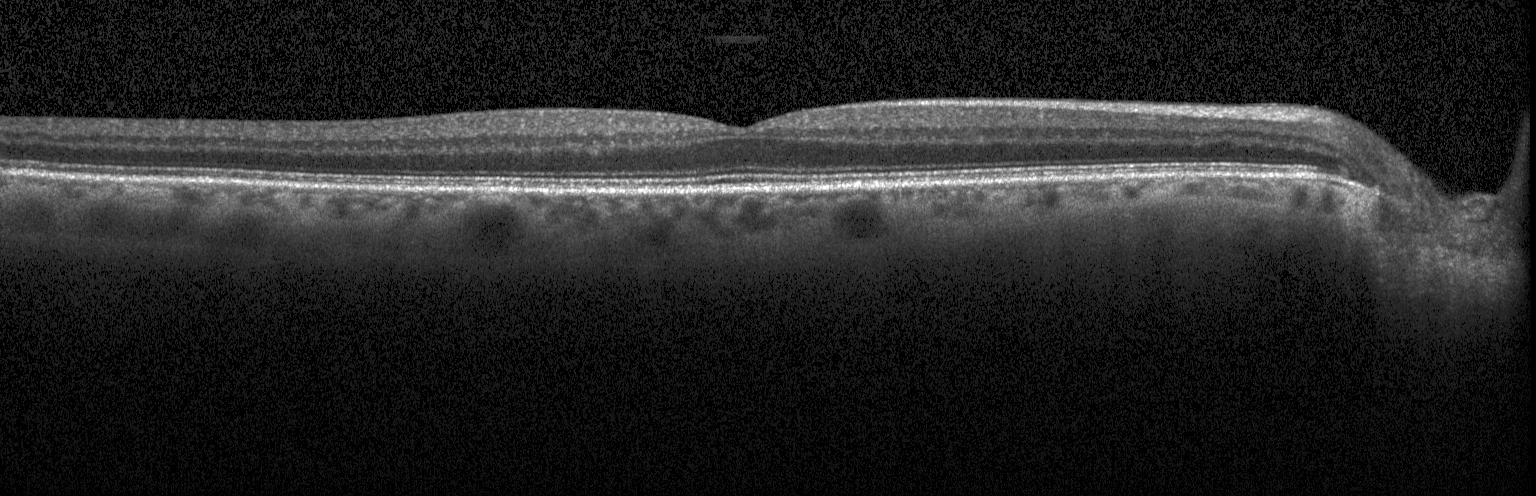
Fovea-centered; SD-OCT; OCT line scan; Heidelberg Spectralis OCT system
Impression: no choroidal neovascularization, diabetic macular edema, or drusen.